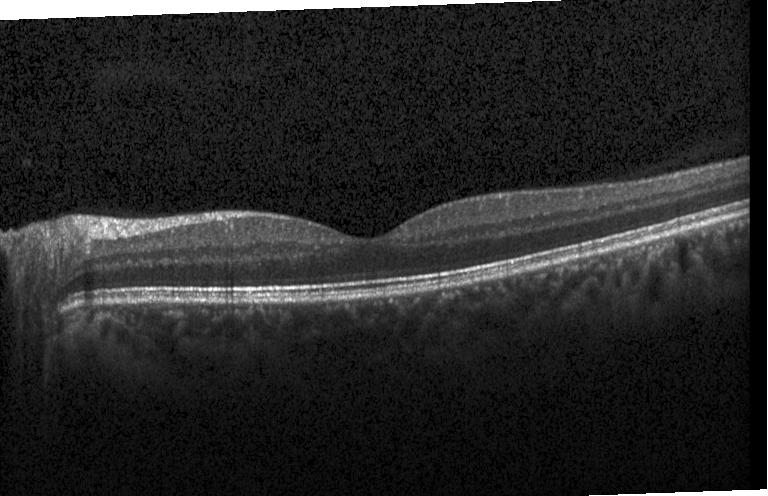

Neither CNV, DME, nor drusen.